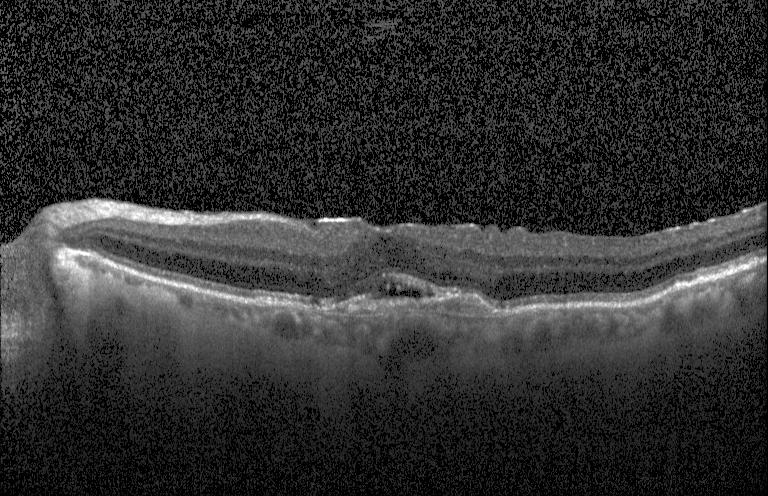 Retinal OCT cross-section.
A choroidal neovascular membrane.